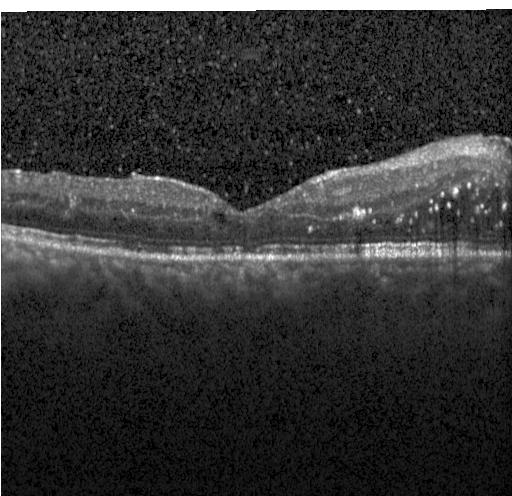
Impression: diabetic macular edema (DME).